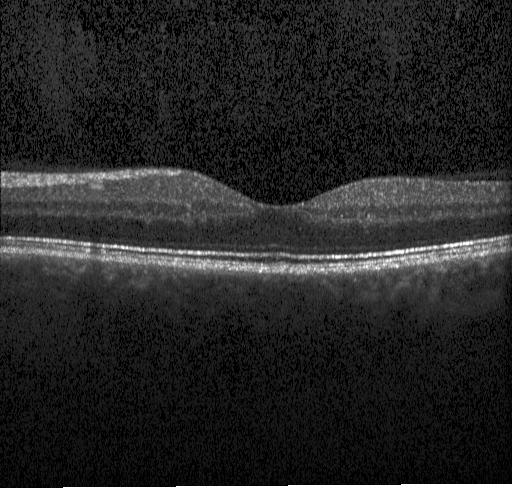
No evidence of choroidal neovascularization, diabetic macular edema, or drusen.